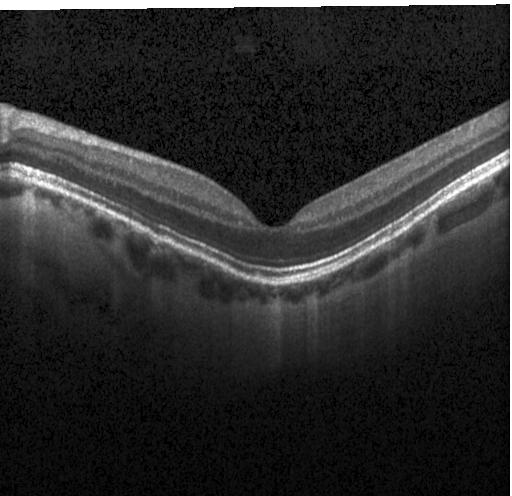 Retinal OCT cross-section.
This B-scan demonstrates no choroidal neovascularization, diabetic macular edema, or drusen.